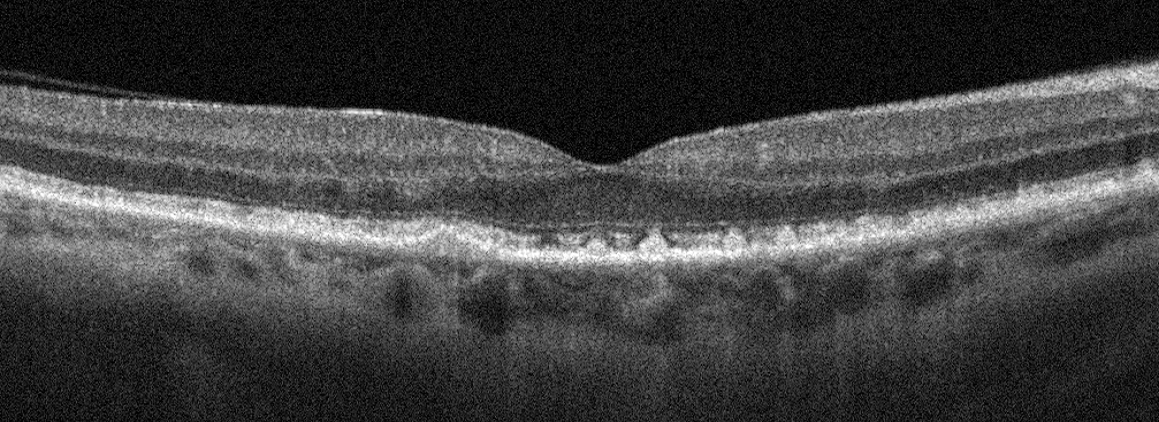

Retinal OCT cross-section, through the macula, right eye. Dx: age-related macular degeneration.